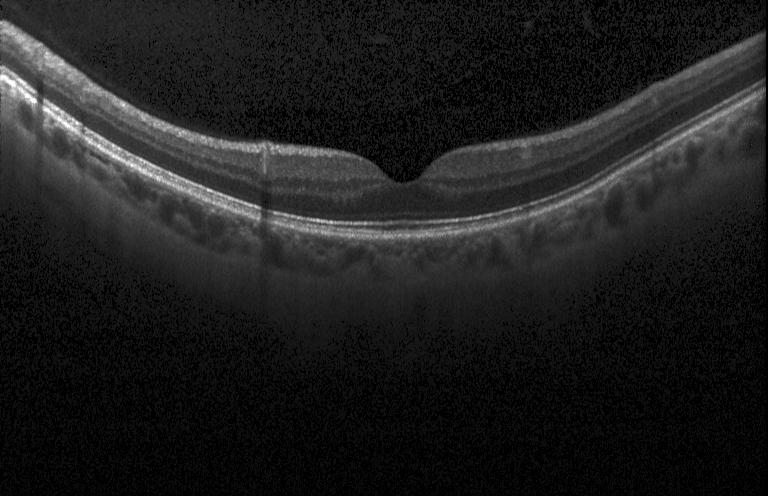 Optical coherence tomography B-scan; SD-OCT; Heidelberg Spectralis.
Finding: no CNV, no DME, and no drusen.